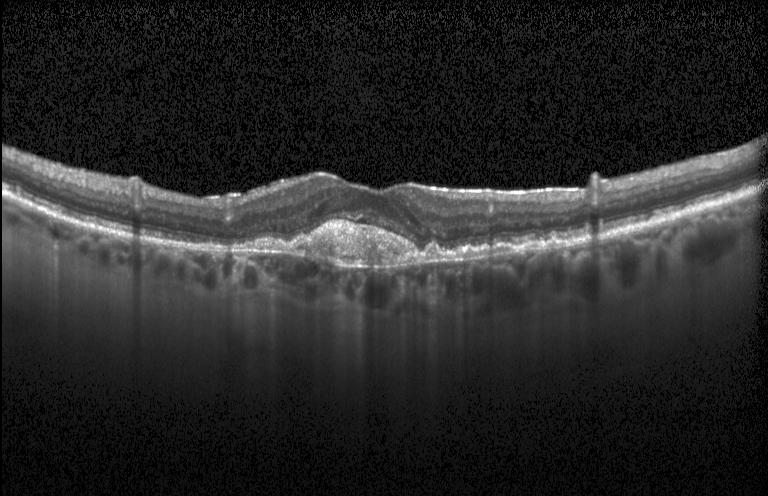

Retinal OCT cross-section, acquired on a Heidelberg Spectralis — OCT finding: CNV.